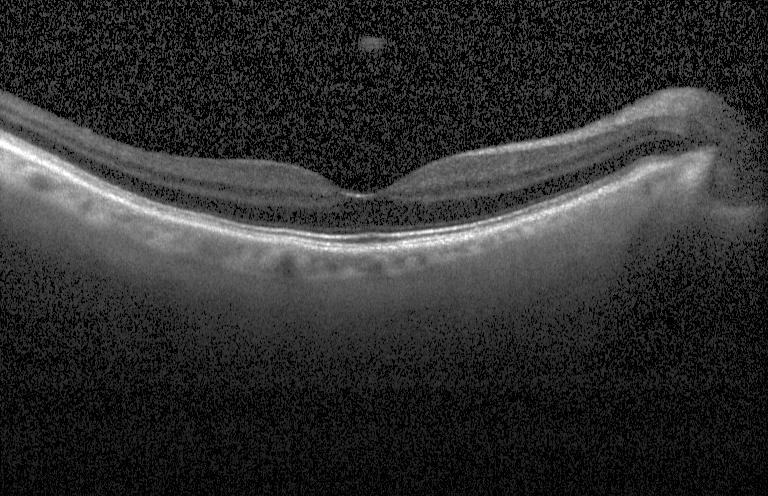
Optical coherence tomography B-scan. This B-scan demonstrates no evidence of CNV, DME, or drusen.